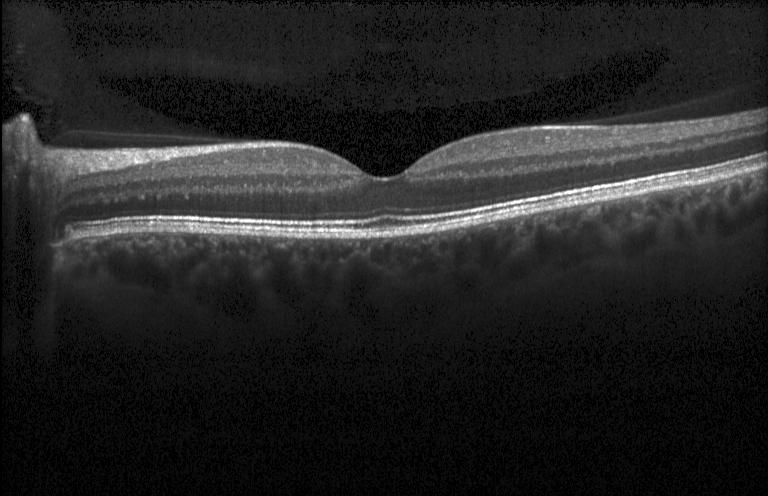
Retinal OCT cross-section, through the macula
OCT finding: no evidence of choroidal neovascularization, diabetic macular edema, or drusen.